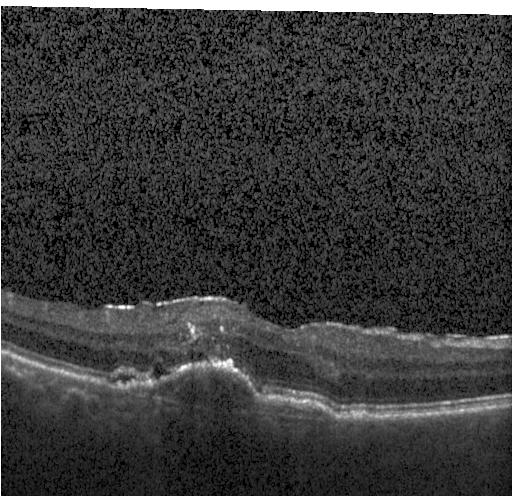
The scan shows choroidal neovascularization (CNV).